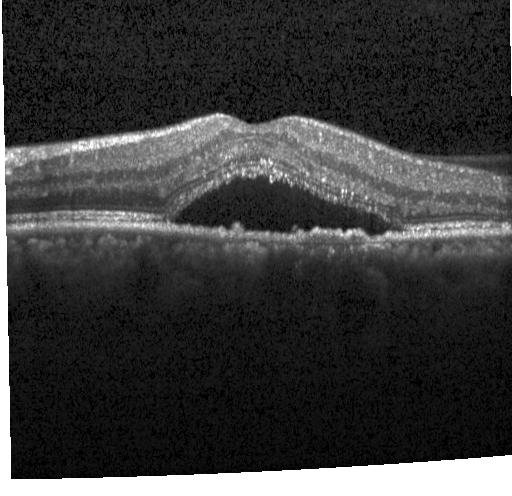 Spectral-domain optical coherence tomography · OCT B-scan. CNV.